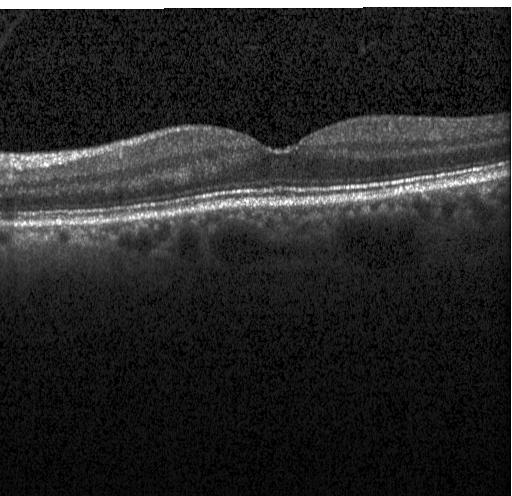
Horizontal scan through the fovea, Heidelberg Spectralis, retinal OCT B-scan — Finding: no choroidal neovascularization, diabetic macular edema, or drusen.